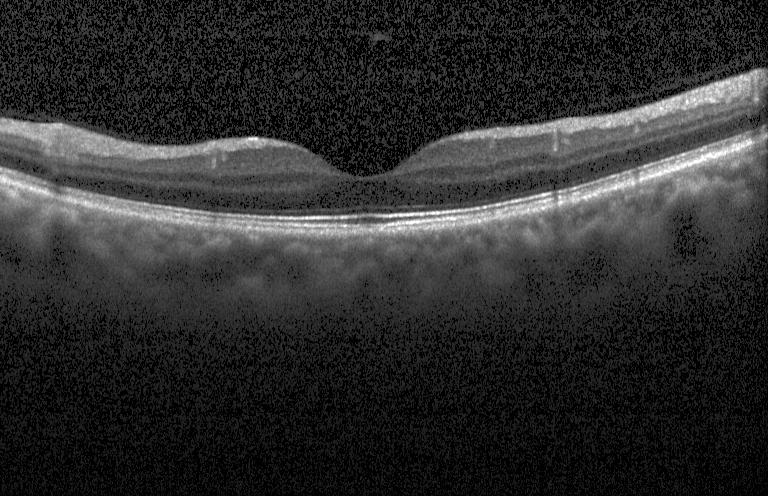 Heidelberg Spectralis, optical coherence tomography B-scan, macular scan, SD-OCT
Impression: no choroidal neovascularization, no diabetic macular edema, and no drusen.